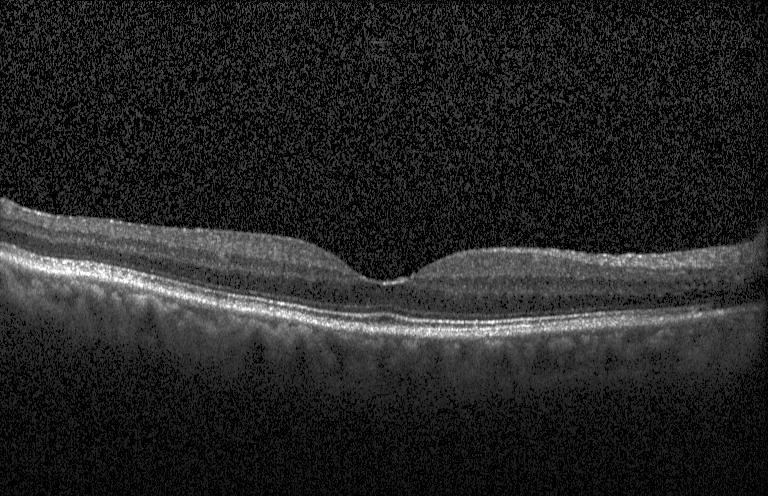
OCT B-scan
This B-scan demonstrates no evidence of CNV, DME, or drusen.